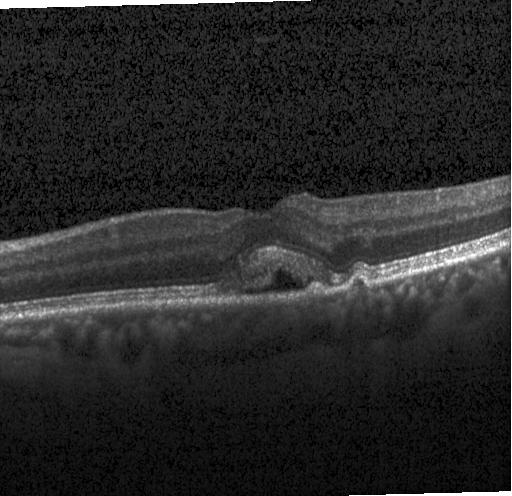 Through the macula; retinal OCT cross-section; spectral-domain OCT — This B-scan demonstrates choroidal neovascularization.